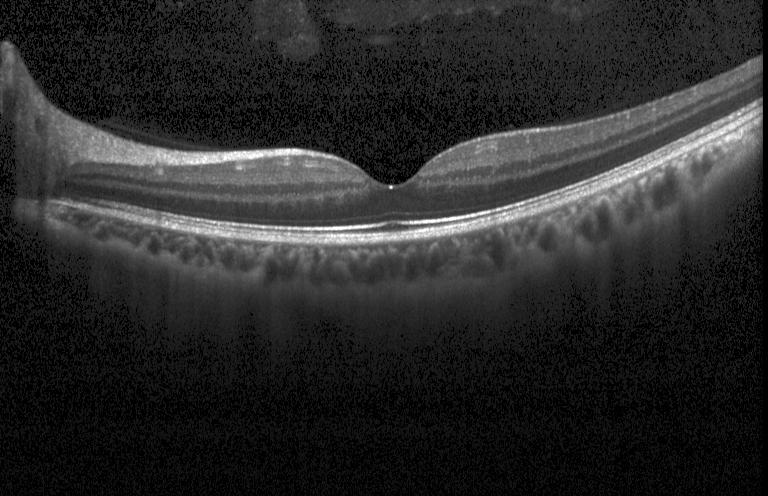
Spectral-domain OCT, optical coherence tomography scan — Assessment: no choroidal neovascularization, no diabetic macular edema, and no drusen.